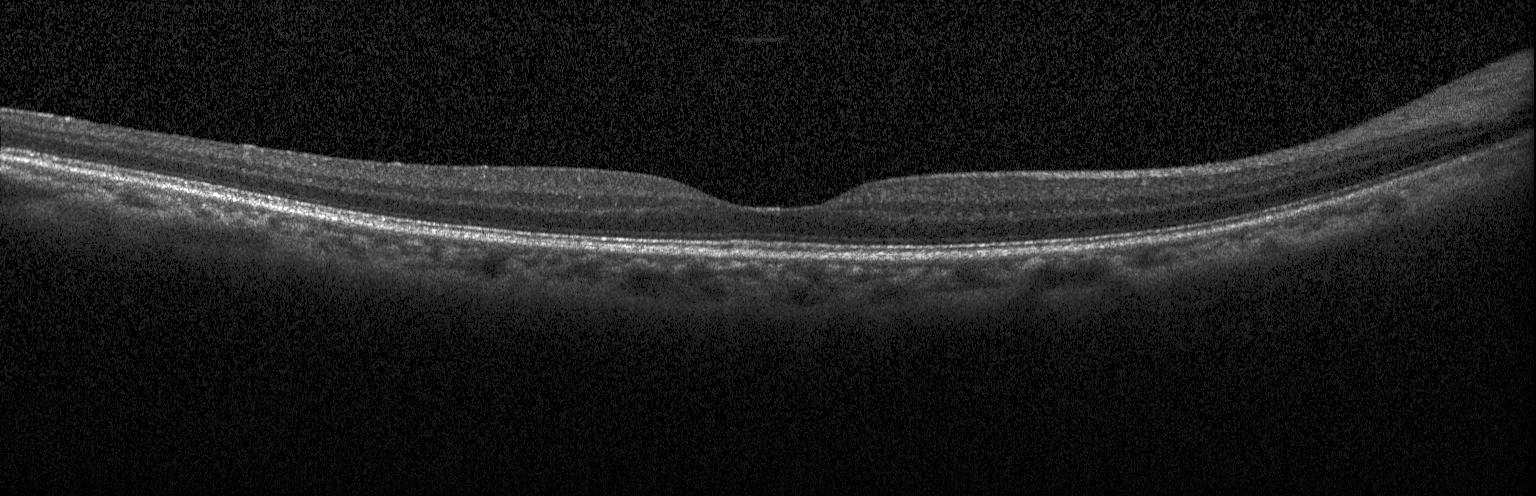 Optical coherence tomography scan
Macular OCT: no CNV, no DME, and no drusen.